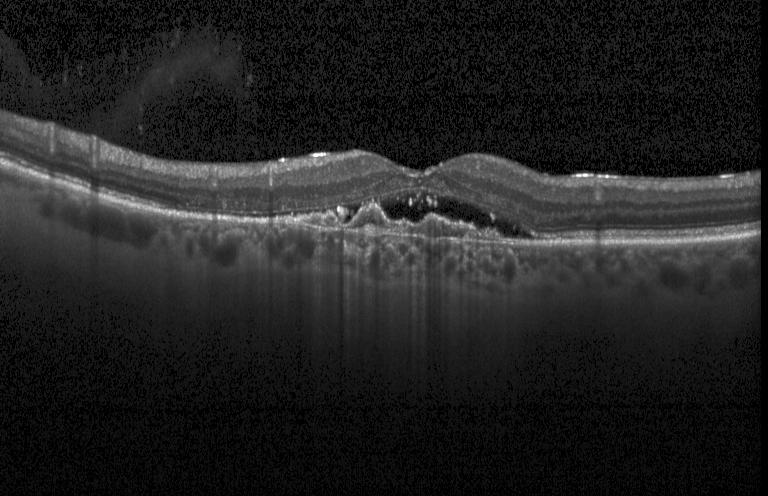 OCT line scan — Macular OCT: a choroidal neovascular membrane.